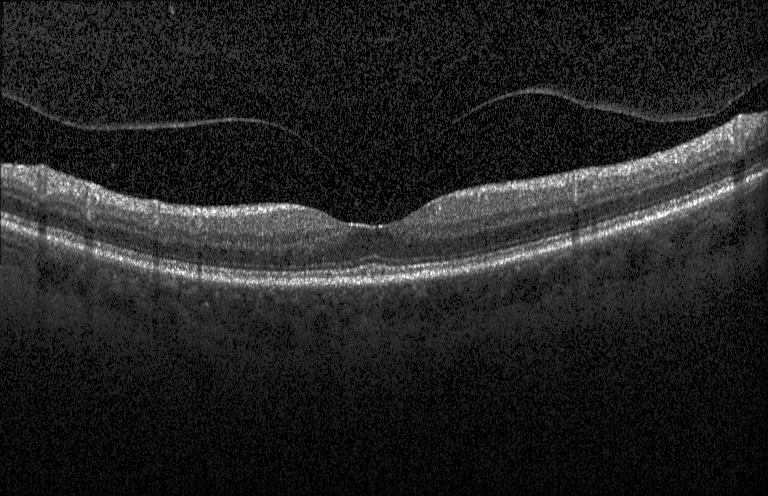 SD-OCT; retinal OCT cross-section; macular scan. Impression: no evidence of CNV, DME, or drusen.